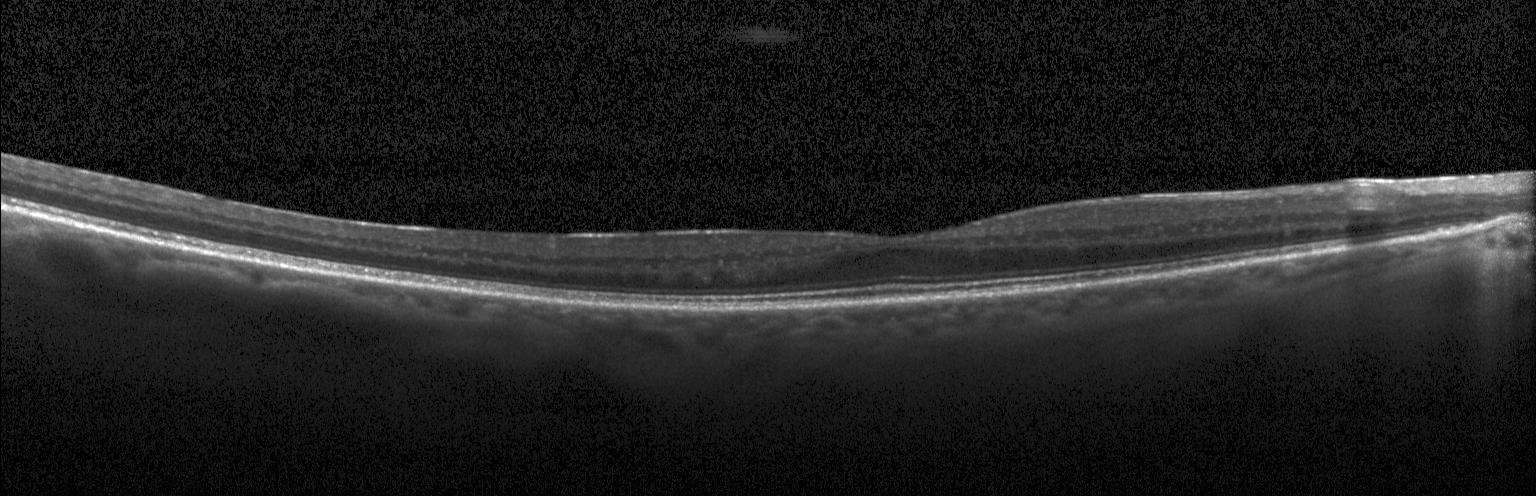

Impression: no choroidal neovascularization, diabetic macular edema, or drusen.